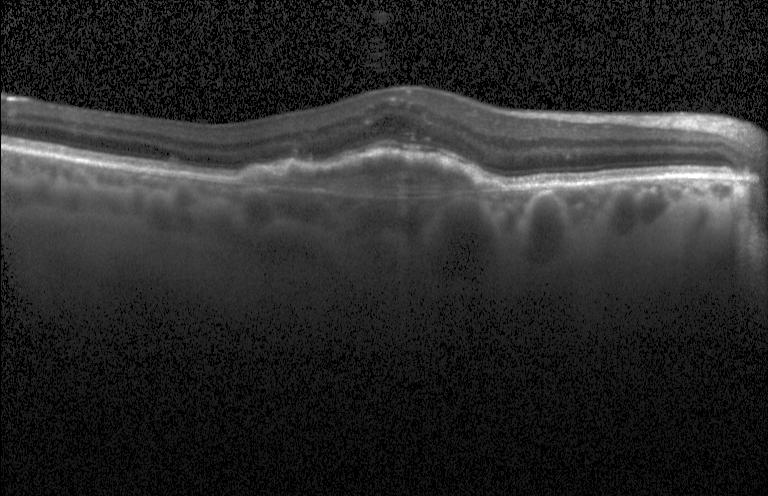
OCT line scan.
Macular OCT: choroidal neovascularization.